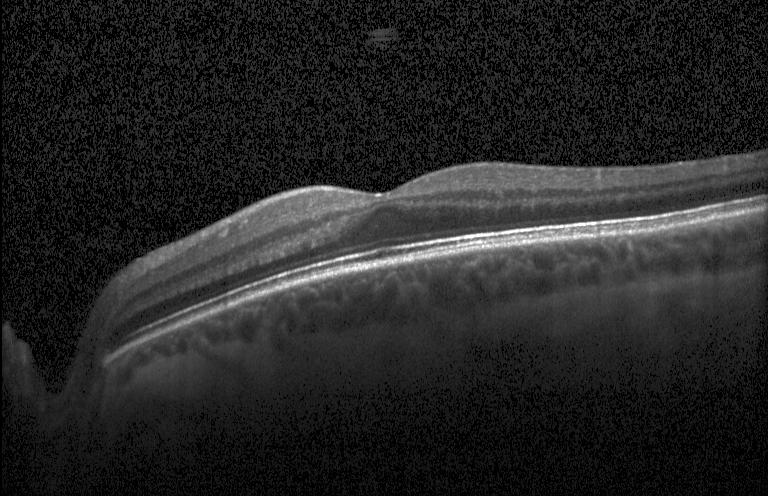 Diagnosis: no choroidal neovascularization, no diabetic macular edema, and no drusen.